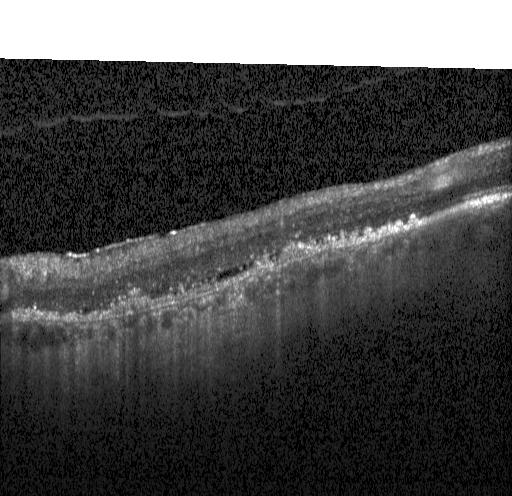

Macular OCT: a choroidal neovascular membrane.